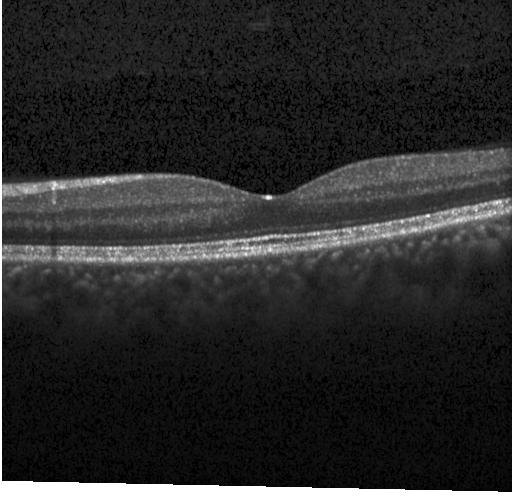 The scan shows no choroidal neovascularization, diabetic macular edema, or drusen.